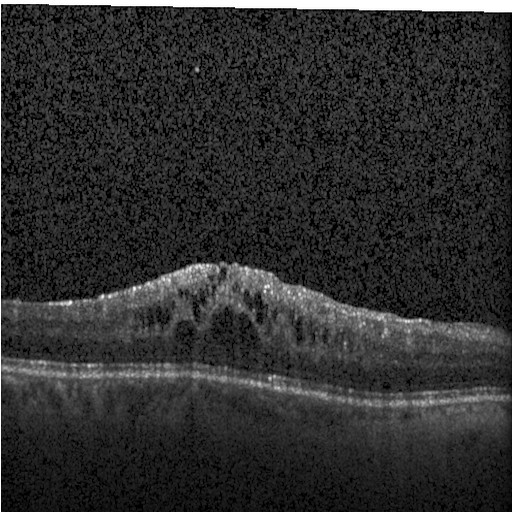
Instrument: Heidelberg Spectralis, centered on the fovea, retinal OCT cross-section.
Dx: diabetic macular edema (DME).